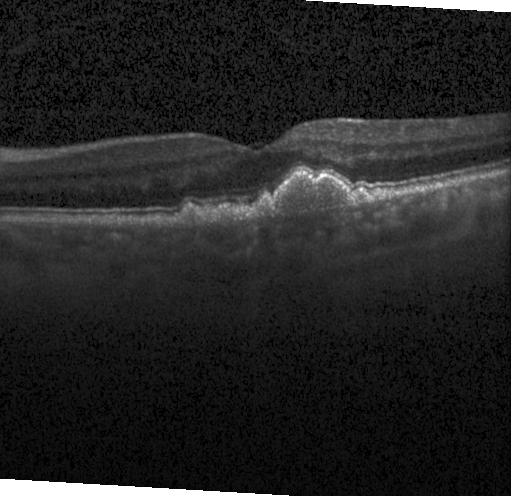 OCT finding: a choroidal neovascular membrane.